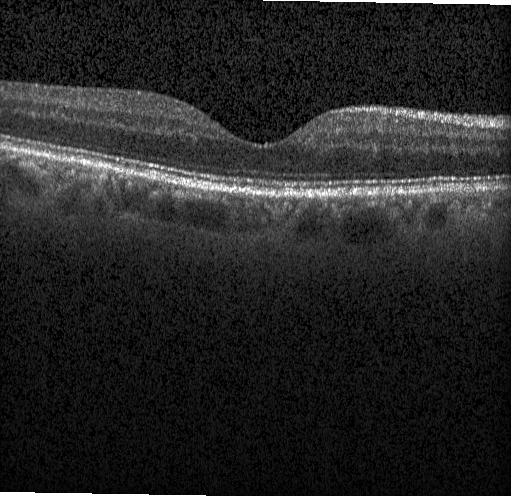

Optical coherence tomography B-scan.
OCT finding: neither CNV, DME, nor drusen.